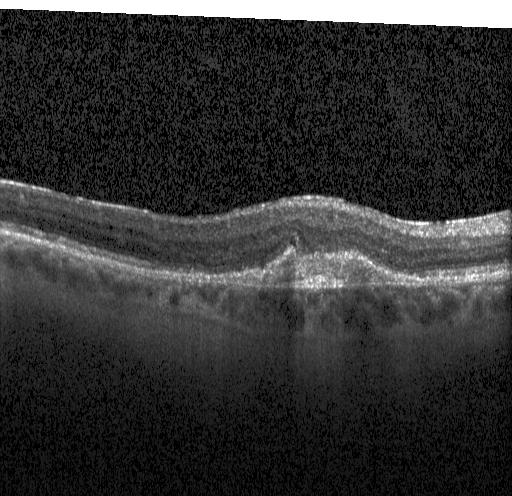 SD-OCT, optical coherence tomography B-scan, macular scan, instrument: Heidelberg Spectralis. A choroidal neovascular membrane.